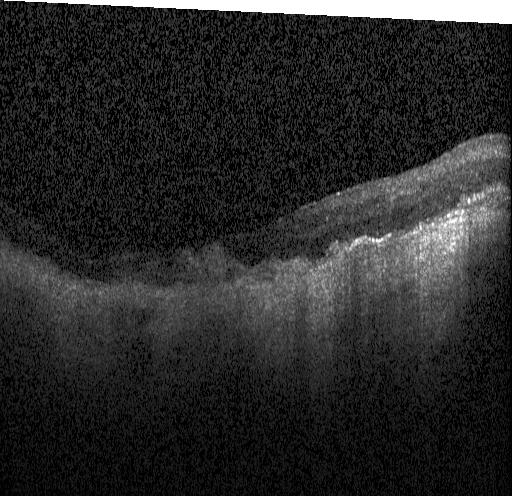
Spectral-domain OCT. Centered on the fovea. Retinal OCT B-scan — Diagnosis: choroidal neovascularization.